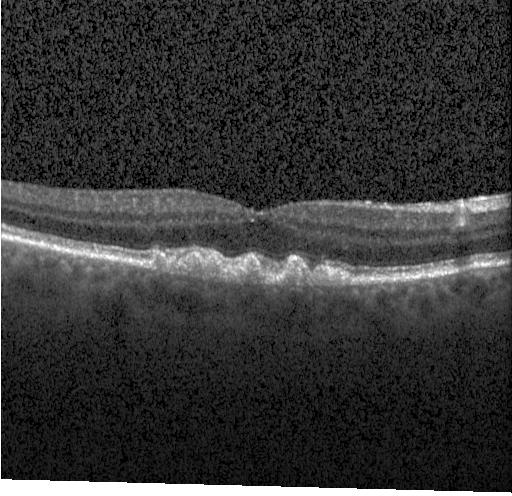

Finding: multiple drusen.